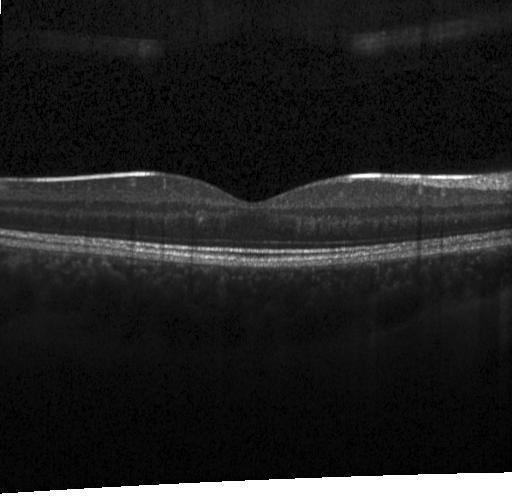 OCT line scan — Diagnosis: no evidence of choroidal neovascularization, diabetic macular edema, or drusen.